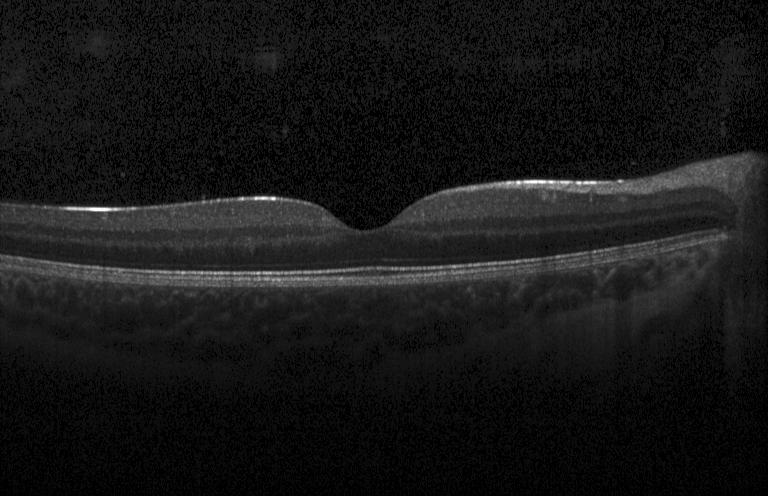
Spectral-domain OCT B-scan: neither choroidal neovascularization, diabetic macular edema, nor drusen.